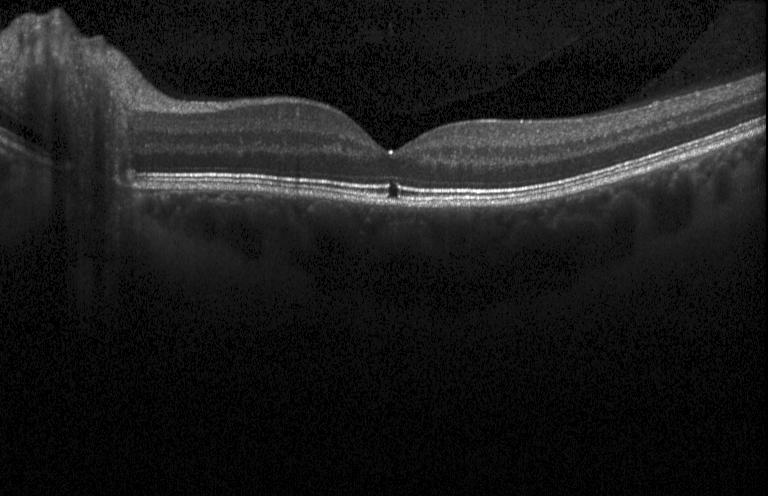

Spectral-domain OCT, optical coherence tomography B-scan. Impression: no choroidal neovascularization, no diabetic macular edema, and no drusen.